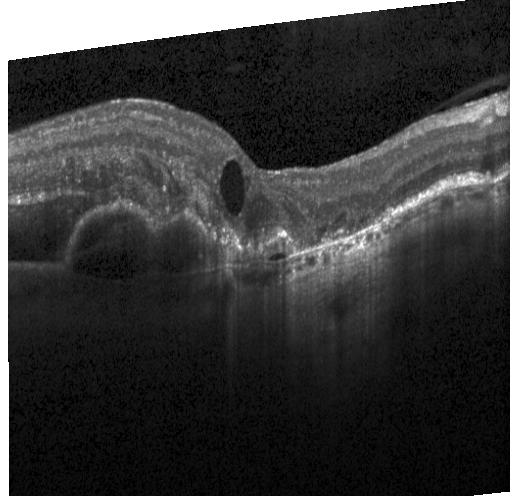

Heidelberg Spectralis OCT system; OCT line scan; SD-OCT. Impression: a choroidal neovascular membrane.